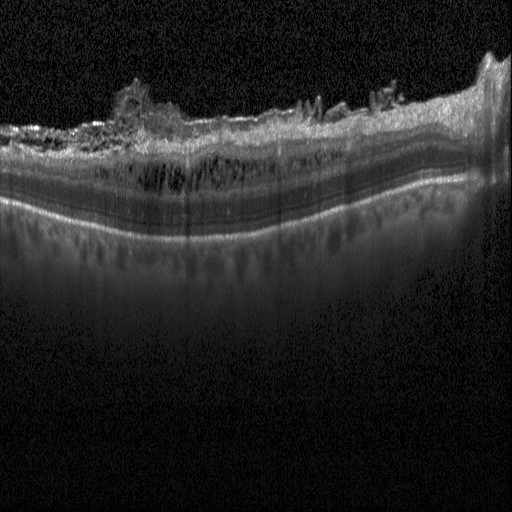

Horizontal scan through the fovea; retinal OCT cross-section; Heidelberg Spectralis OCT system; spectral-domain OCT — DME.